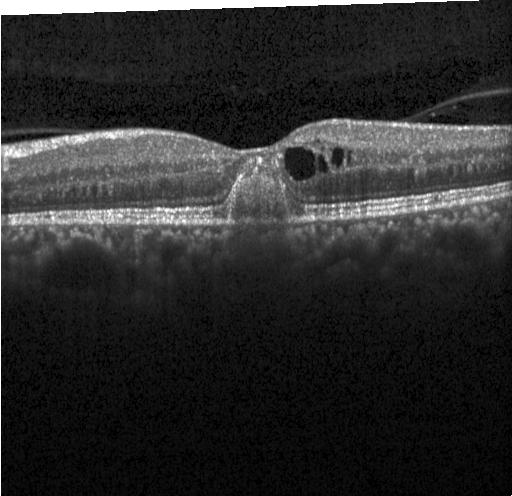

SD-OCT, acquired on a Heidelberg Spectralis, fovea-centered, OCT line scan.
Diagnosis: a choroidal neovascular membrane.